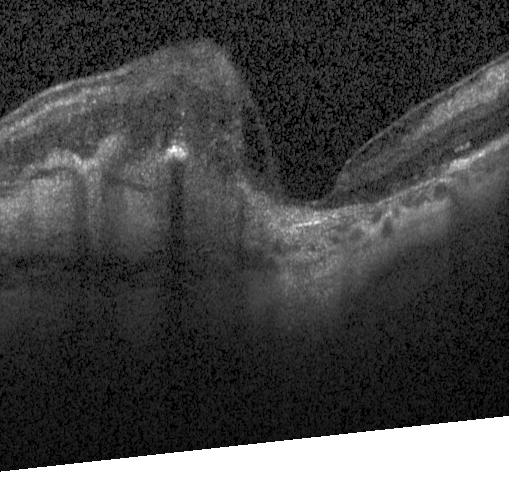

Finding: a choroidal neovascular membrane.